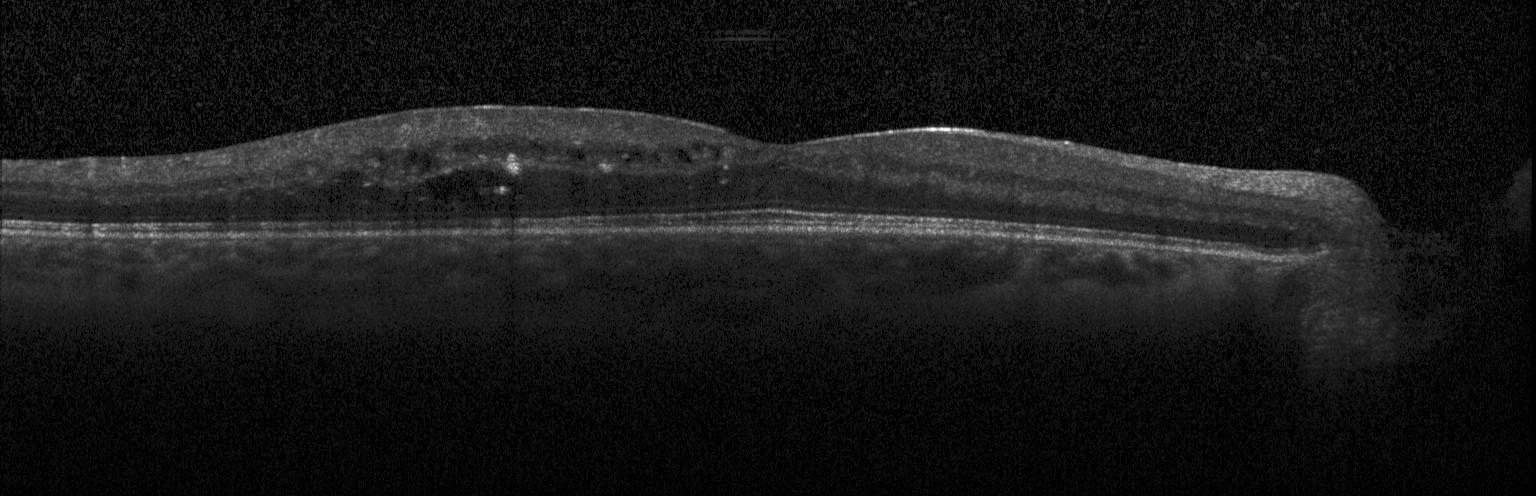 Impression: diabetic macular edema (DME).